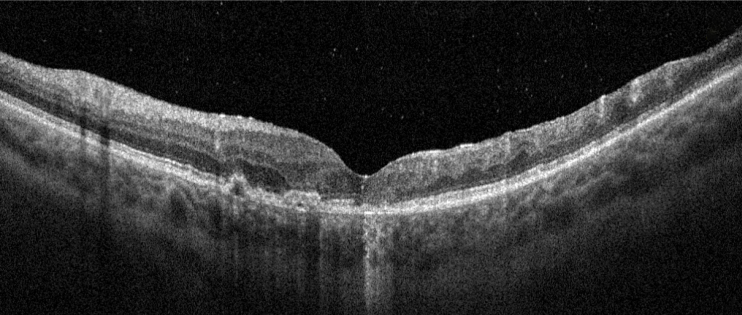
Optical coherence tomography B-scan.
Assessment: diabetic macular edema.